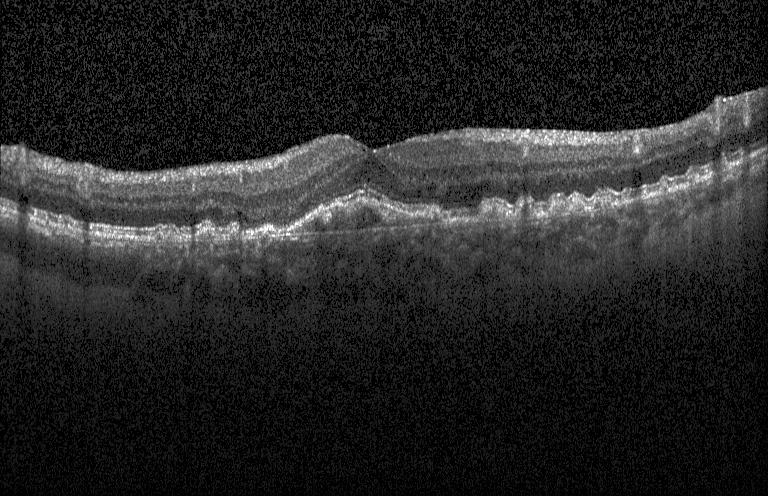

Spectral-domain optical coherence tomography, optical coherence tomography B-scan. CNV.